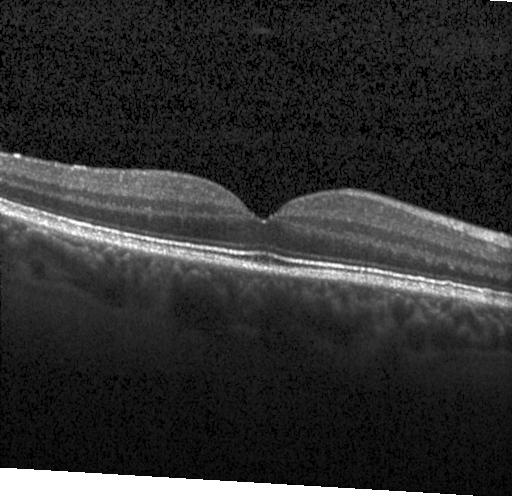 OCT B-scan; instrument: Heidelberg Spectralis; SD-OCT
Assessment: neither CNV, DME, nor drusen.